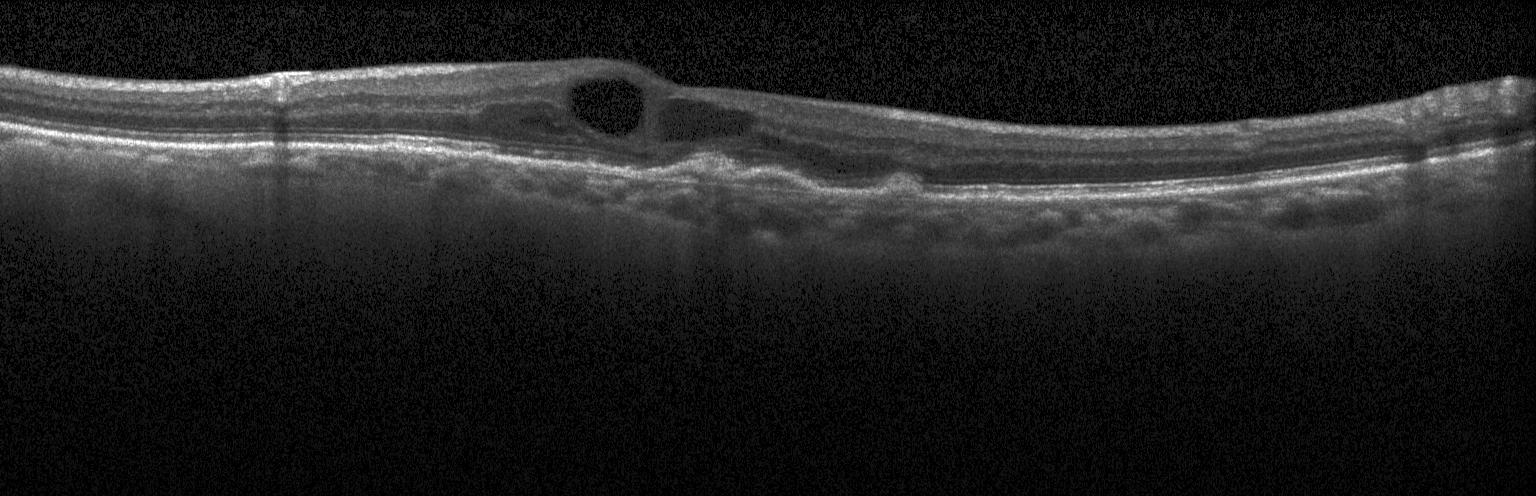
Optical coherence tomography B-scan. Through the macula. Spectral-domain optical coherence tomography. Diagnosis: a choroidal neovascular membrane.